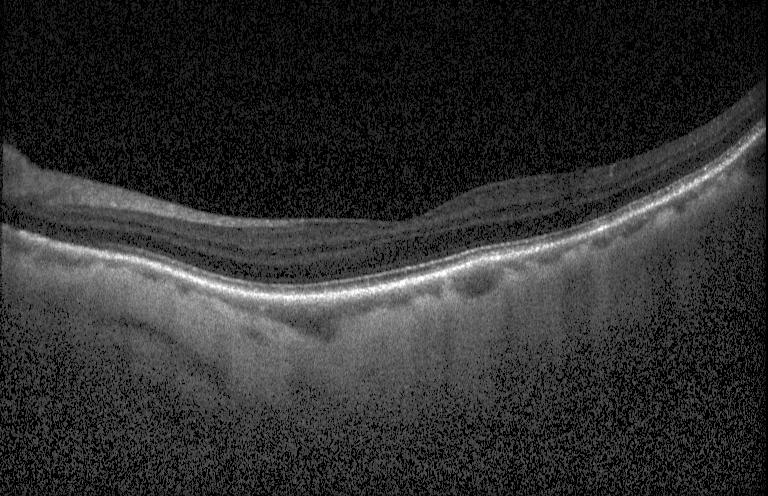

OCT B-scan — Impression: no choroidal neovascularization, no diabetic macular edema, and no drusen.